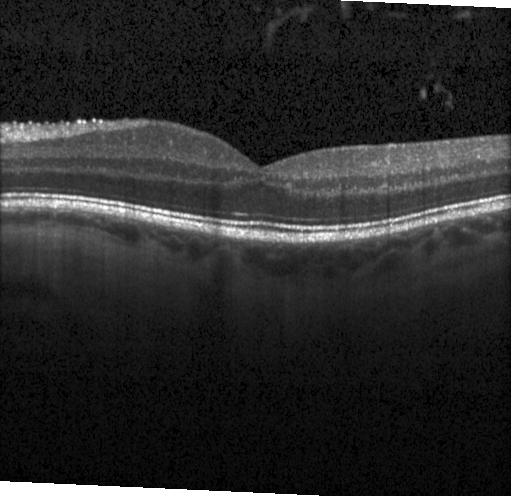

OCT B-scan showing no evidence of choroidal neovascularization, diabetic macular edema, or drusen.